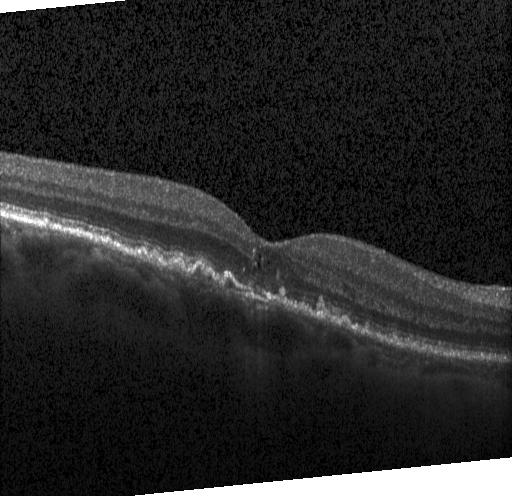 Impression: sub-RPE drusenoid deposits.